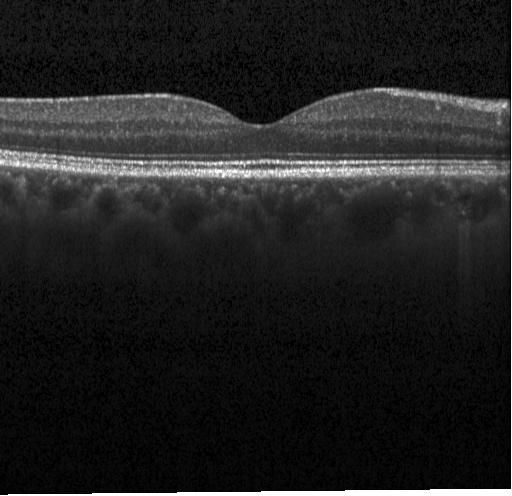
Spectral-domain optical coherence tomography; retinal OCT B-scan. The scan shows no choroidal neovascularization, diabetic macular edema, or drusen.